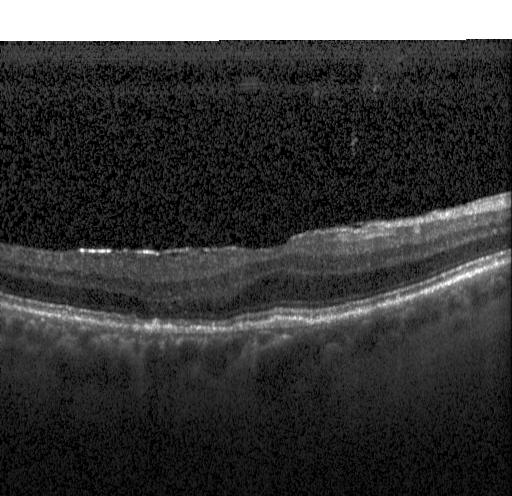

Optical coherence tomography scan. Horizontal scan through the fovea. Diagnosis: choroidal neovascularization (CNV).